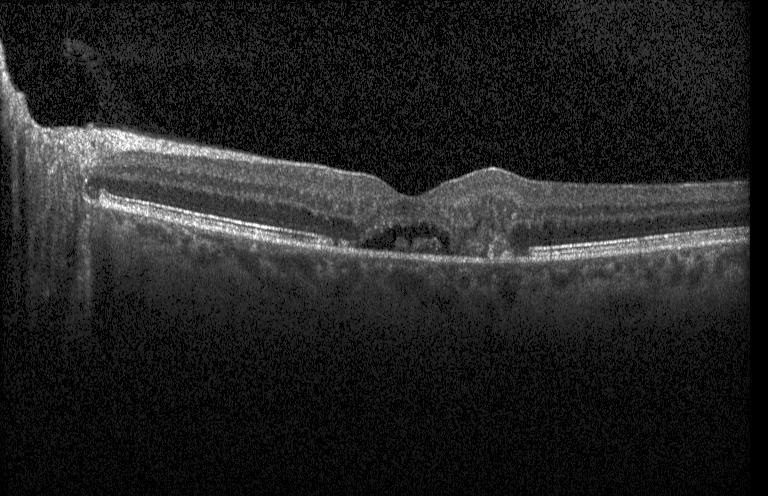
SD-OCT · retinal OCT cross-section
Assessment: choroidal neovascularization (CNV).